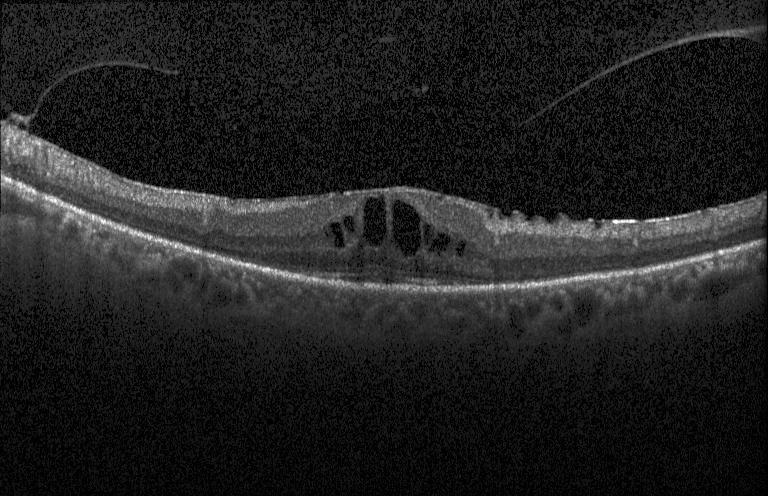

Horizontal scan through the fovea, optical coherence tomography B-scan, Heidelberg Spectralis OCT system. Impression: diabetic macular edema (DME).